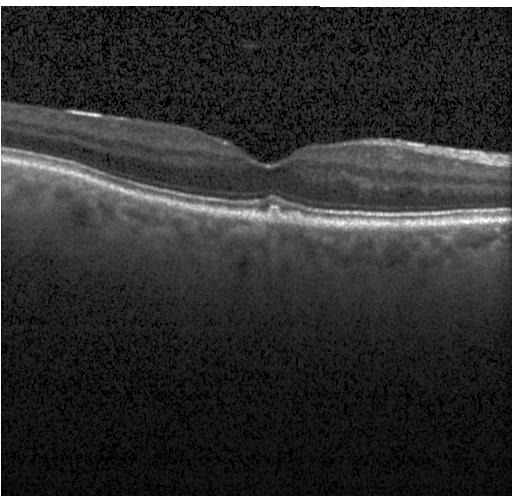 OCT B-scan, acquired on a Heidelberg Spectralis, spectral-domain optical coherence tomography.
Impression: multiple drusen.